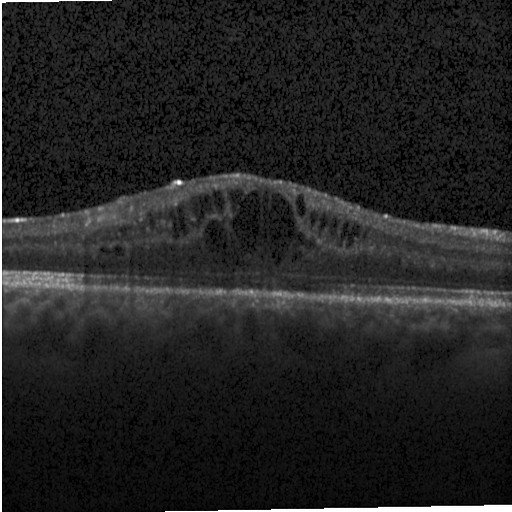 Optical coherence tomography B-scan; macular scan
Assessment: diabetic macular edema (DME).